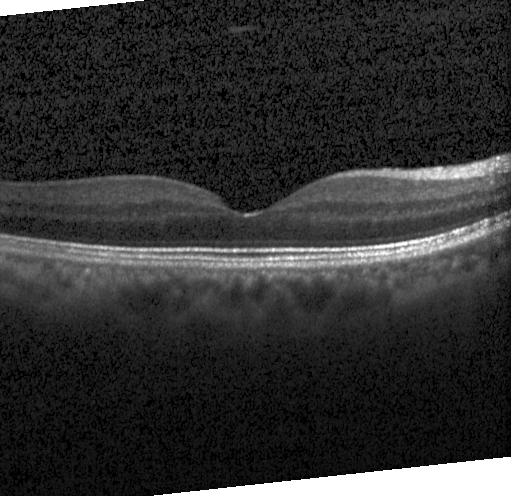
Spectral-domain OCT, Heidelberg Spectralis, OCT B-scan, fovea-centered — Assessment: neither choroidal neovascularization, diabetic macular edema, nor drusen.